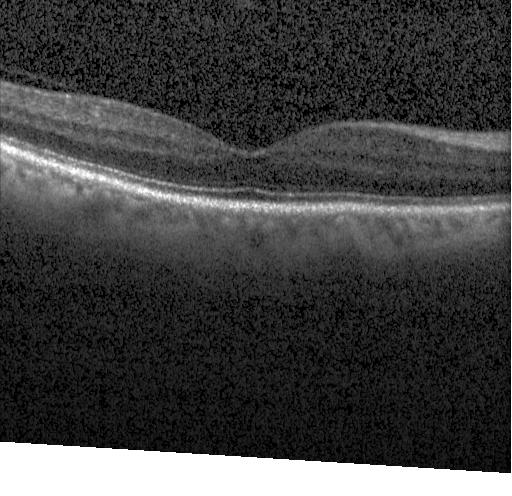 Optical coherence tomography scan; instrument: Heidelberg Spectralis; horizontal scan through the fovea. OCT finding: no choroidal neovascularization, no diabetic macular edema, and no drusen.